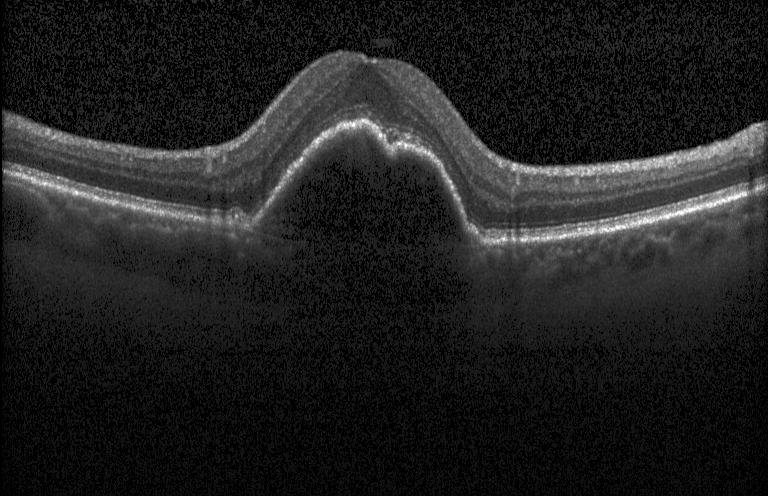 Macular OCT: CNV.